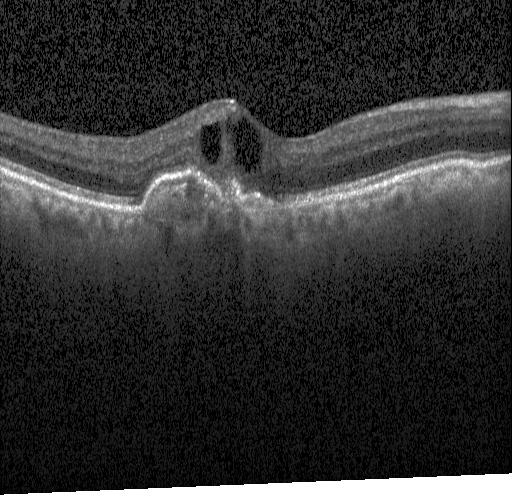

Heidelberg Spectralis OCT system, spectral-domain optical coherence tomography, retinal OCT B-scan. The scan shows a choroidal neovascular membrane.